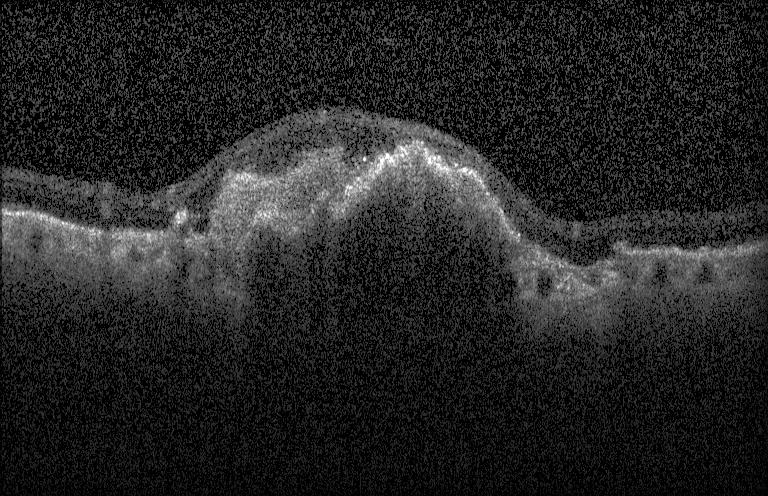

A choroidal neovascular membrane.